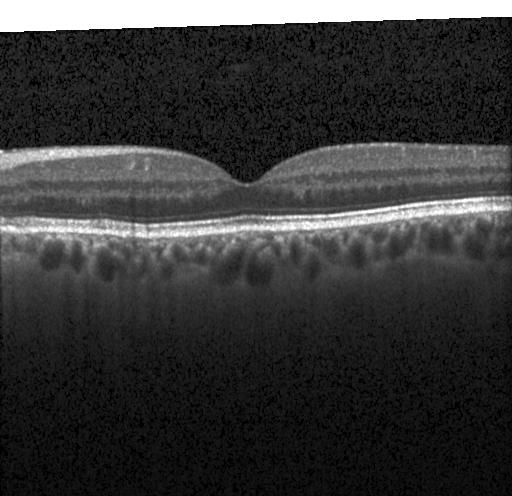
Retinal OCT cross-section showing neither choroidal neovascularization, diabetic macular edema, nor drusen.